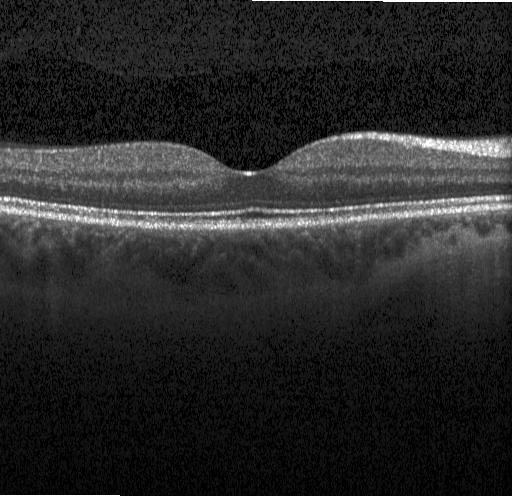
Macular OCT: no choroidal neovascularization, no diabetic macular edema, and no drusen.